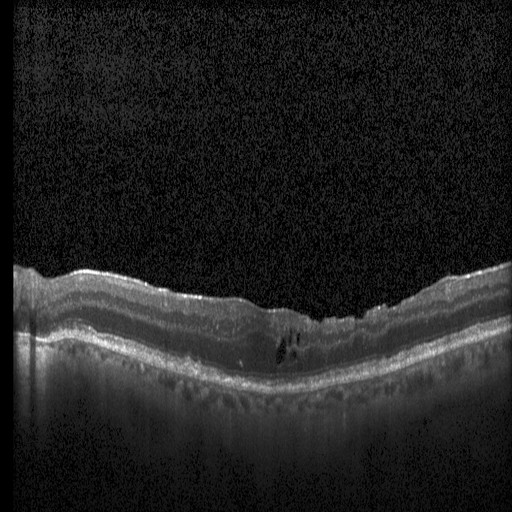 Heidelberg Spectralis OCT system; centered on the fovea; retinal OCT cross-section; spectral-domain optical coherence tomography.
Dx: diabetic macular edema.